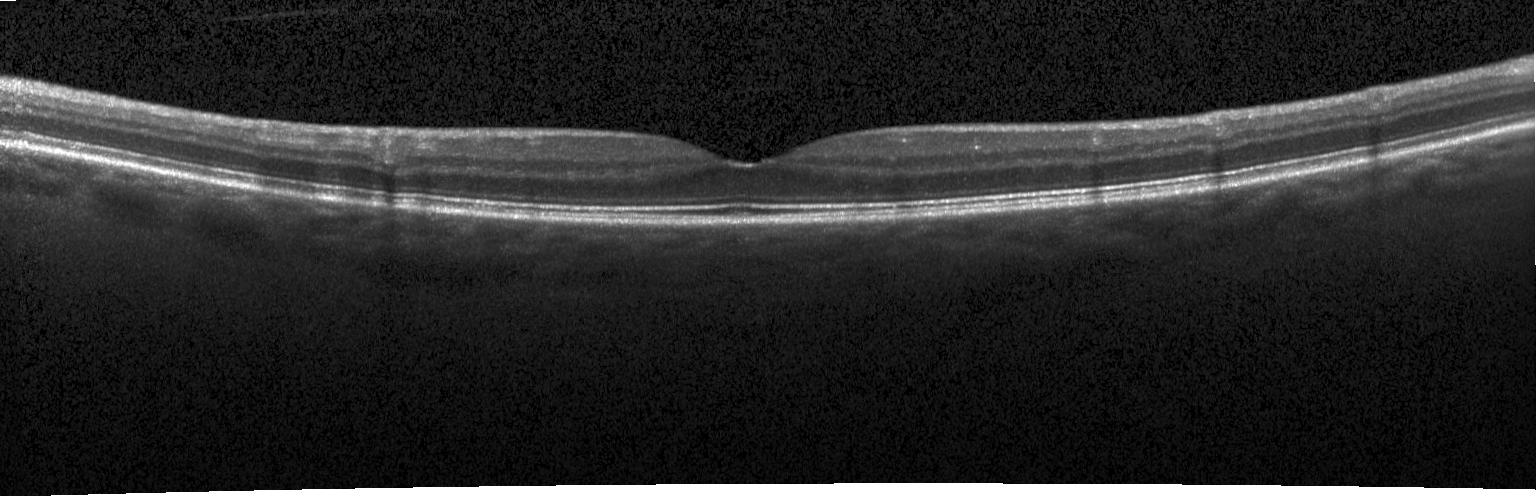
Retinal OCT cross-section — Dx: no choroidal neovascularization, no diabetic macular edema, and no drusen.